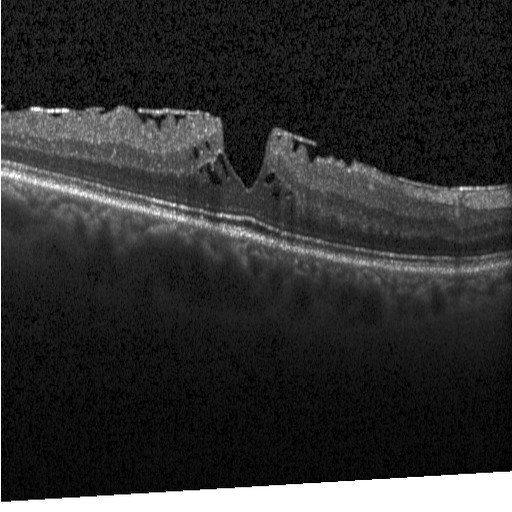

Assessment: diabetic macular edema (DME).